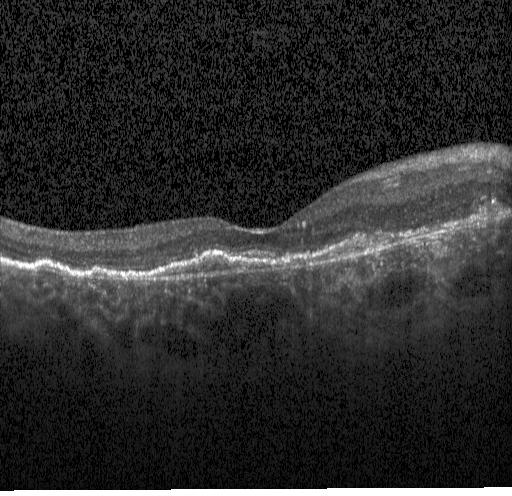

Impression: a choroidal neovascular membrane.